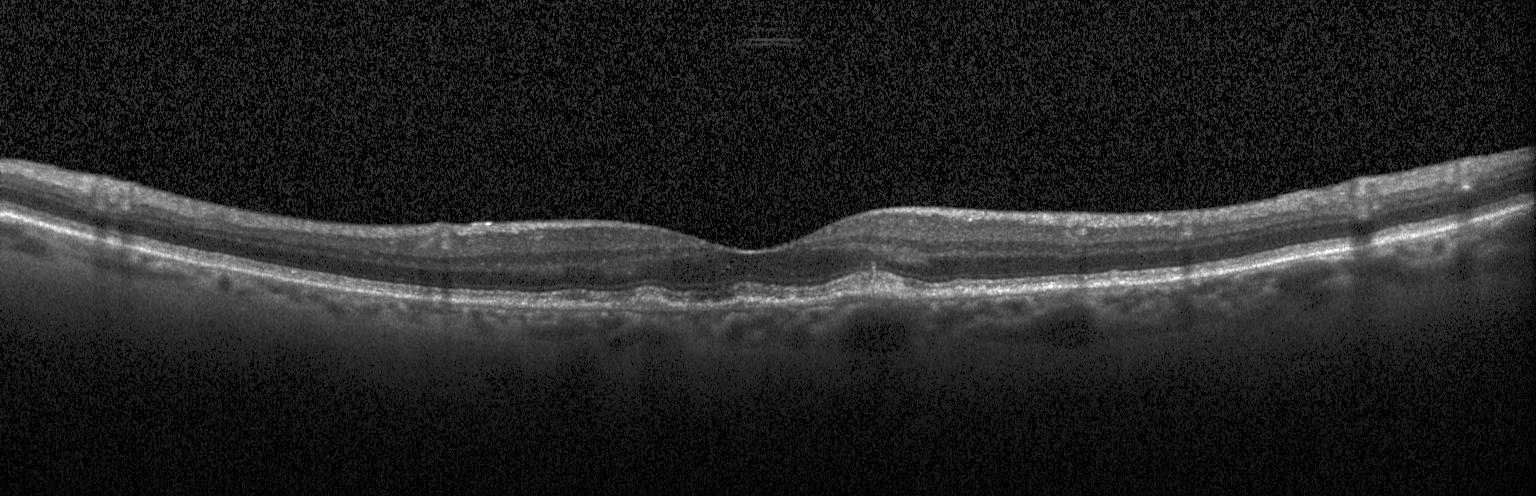

OCT finding: multiple drusen.